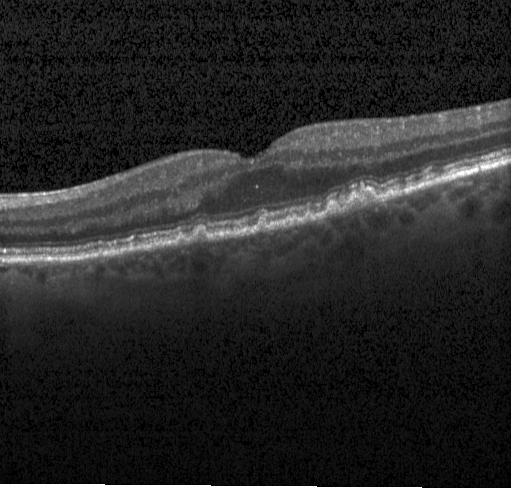
Heidelberg Spectralis OCT system. Optical coherence tomography scan. Spectral-domain optical coherence tomography. Centered on the fovea
Finding: drusen.